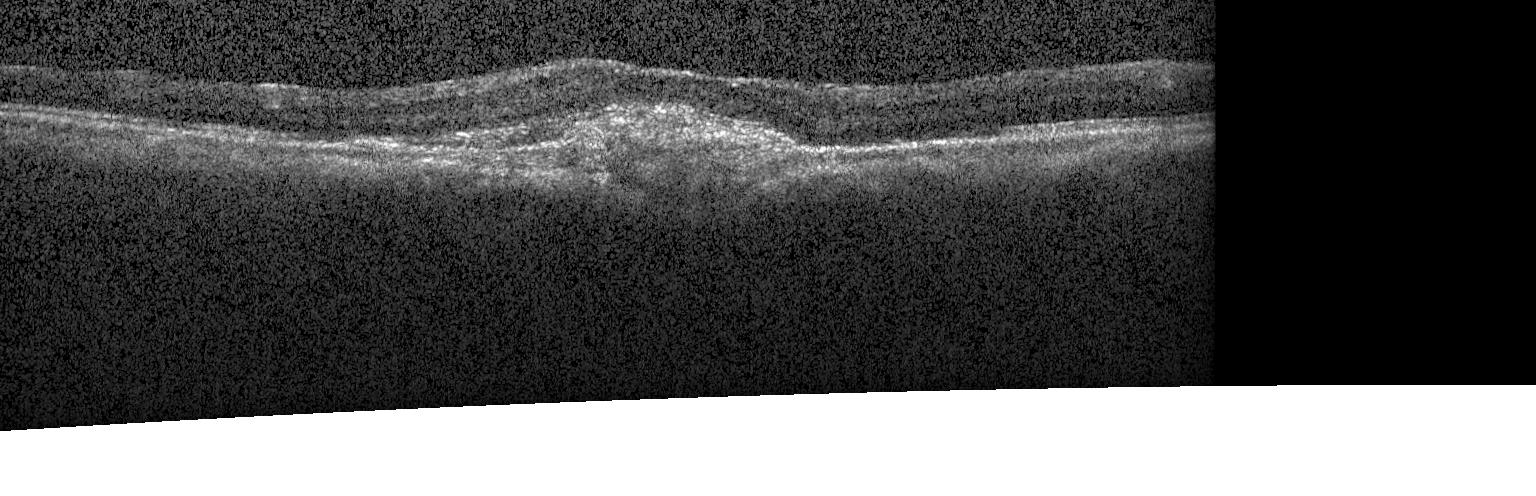 OCT line scan · horizontal scan through the fovea — Dx: a choroidal neovascular membrane.